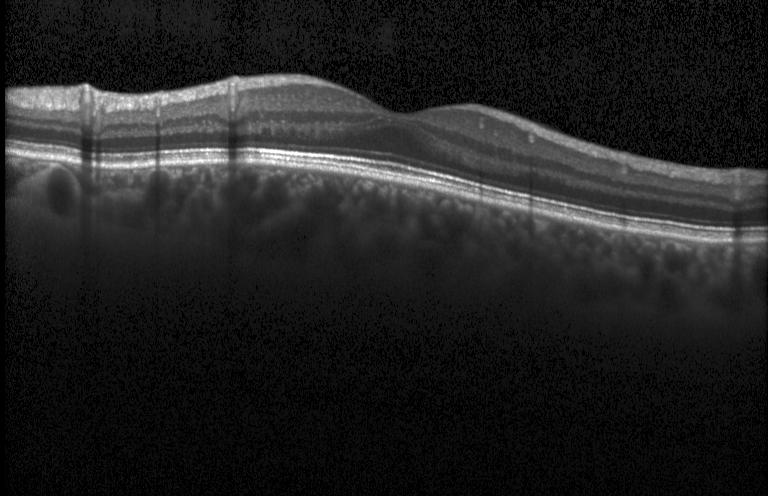
Heidelberg Spectralis OCT system. Spectral-domain OCT. Retinal OCT cross-section.
Finding: no choroidal neovascularization, diabetic macular edema, or drusen.